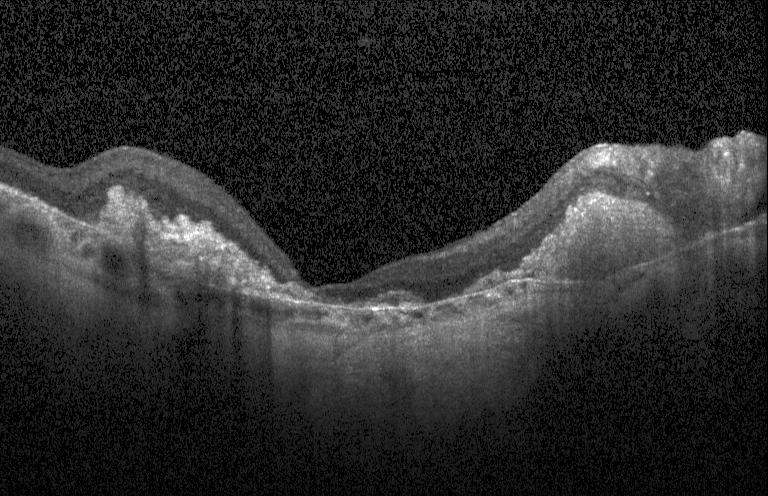

Diagnosis: choroidal neovascularization (CNV).